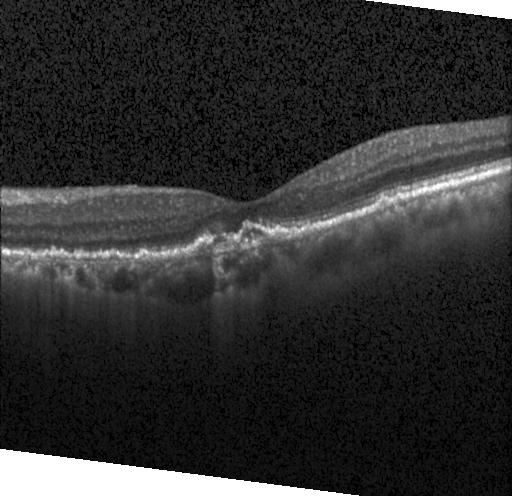 Diagnosis: choroidal neovascularization (CNV).